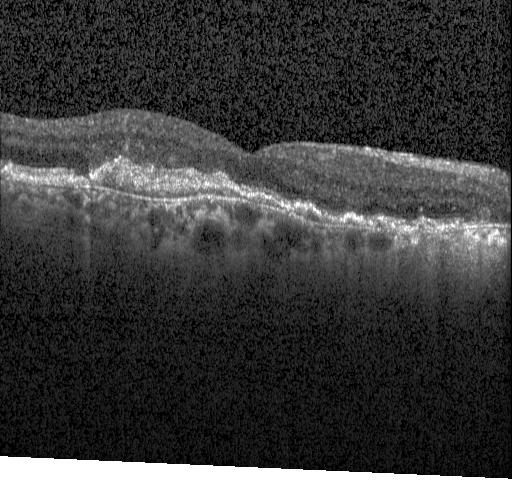 OCT line scan — Finding: a choroidal neovascular membrane.